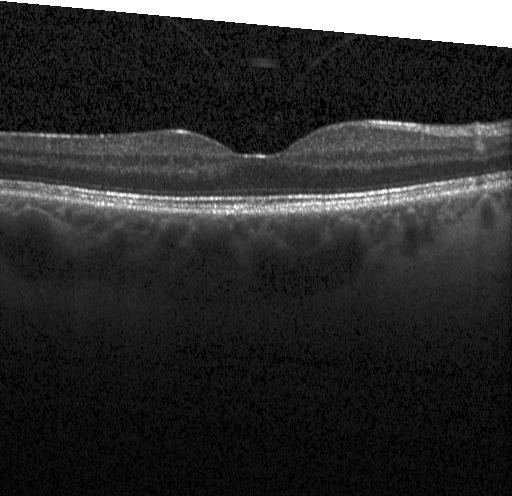 Optical coherence tomography B-scan, through the macula.
Diagnosis: neither choroidal neovascularization, diabetic macular edema, nor drusen.